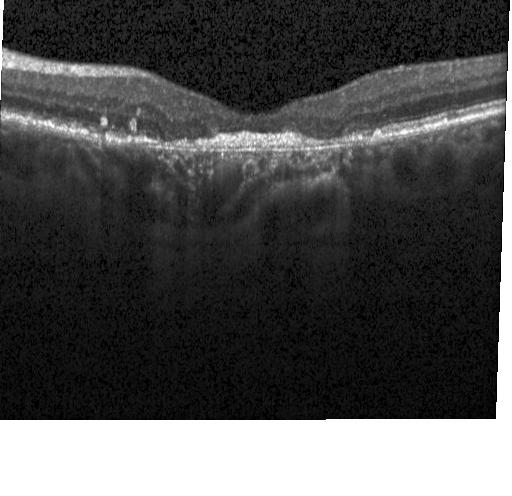

Optical coherence tomography scan — This B-scan demonstrates a choroidal neovascular membrane.